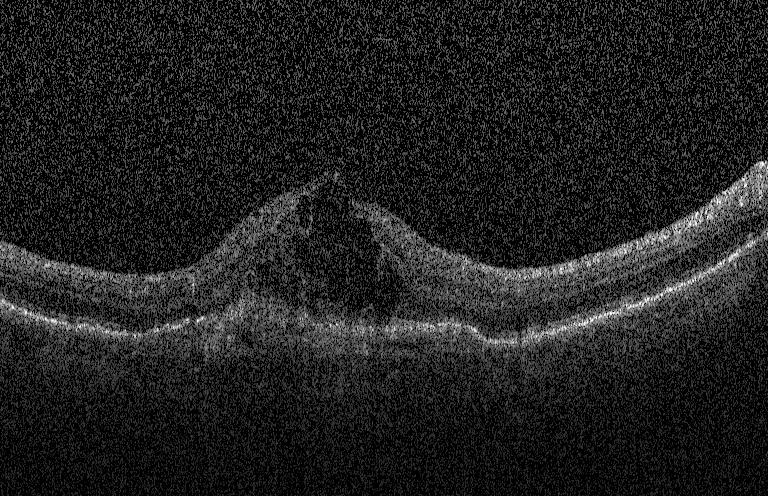

OCT line scan — Assessment: a choroidal neovascular membrane.